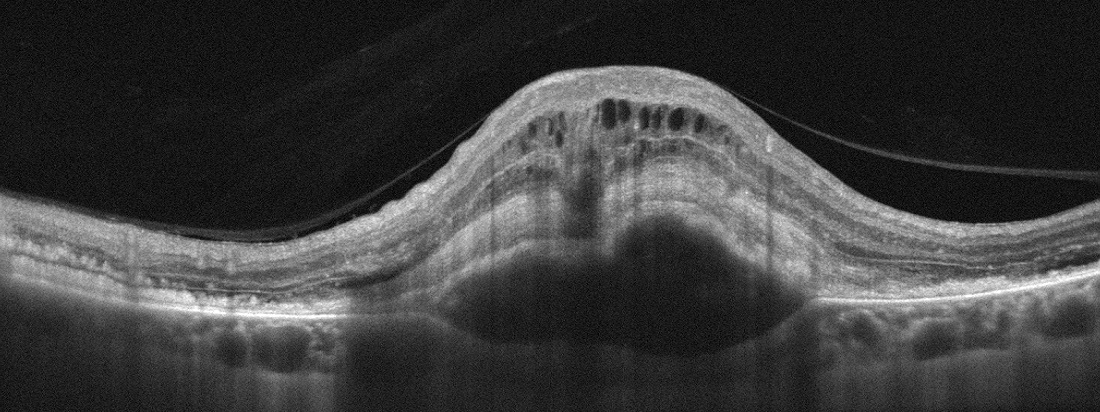
Diagnosis: age-related macular degeneration (AMD).